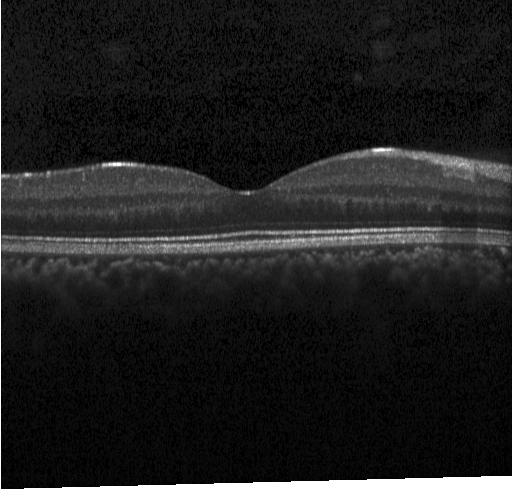 Heidelberg Spectralis OCT system · OCT line scan · spectral-domain OCT — Diagnosis: no evidence of choroidal neovascularization, diabetic macular edema, or drusen.